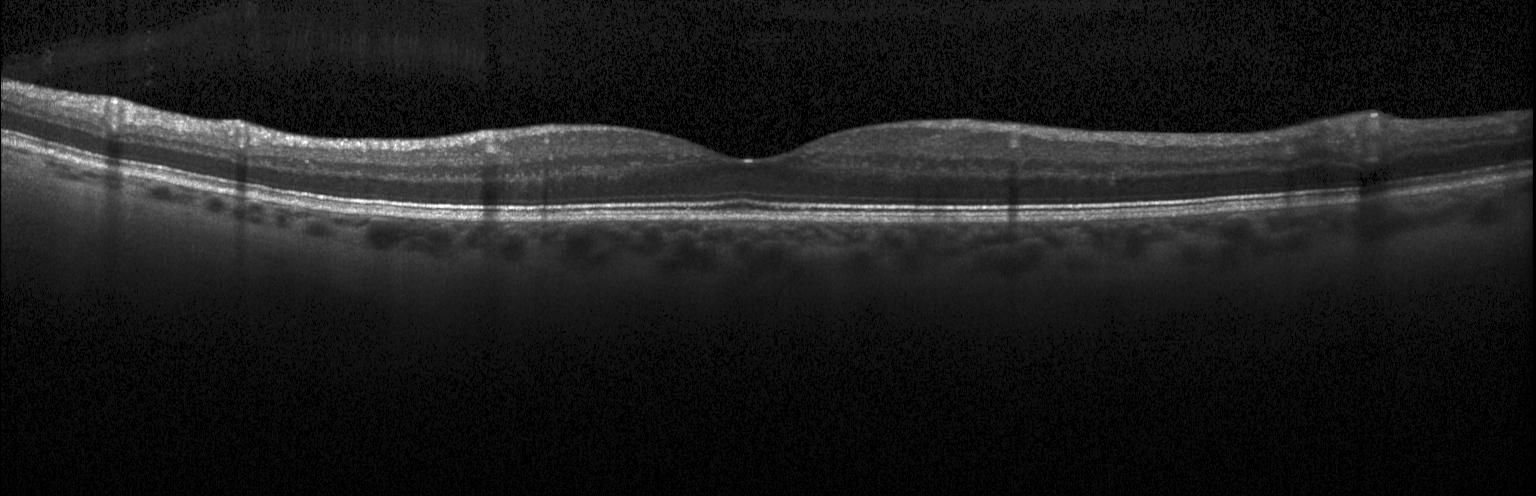 OCT B-scan showing no choroidal neovascularization, diabetic macular edema, or drusen.